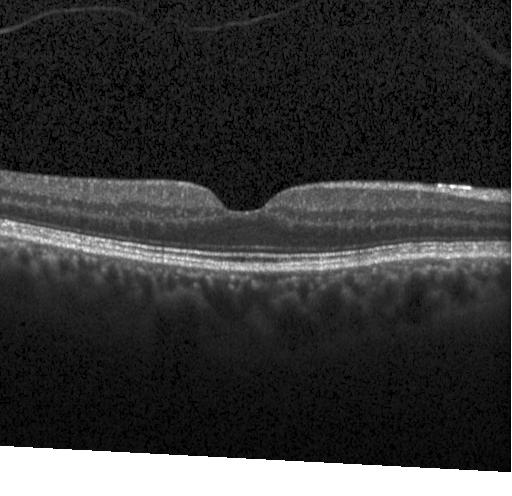 Impression: no CNV, no DME, and no drusen.